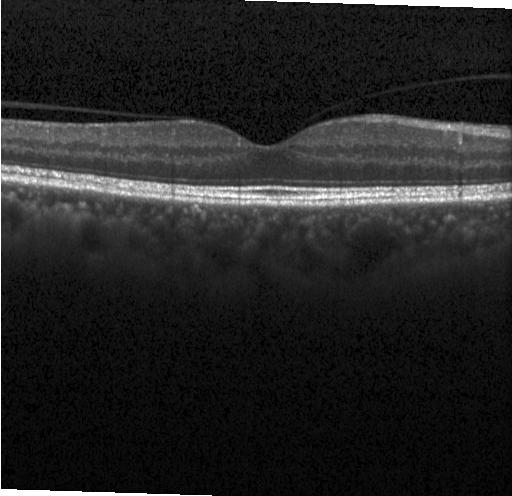
Centered on the fovea, OCT line scan, SD-OCT, Heidelberg Spectralis OCT system — Diagnosis: no CNV, DME, or drusen.